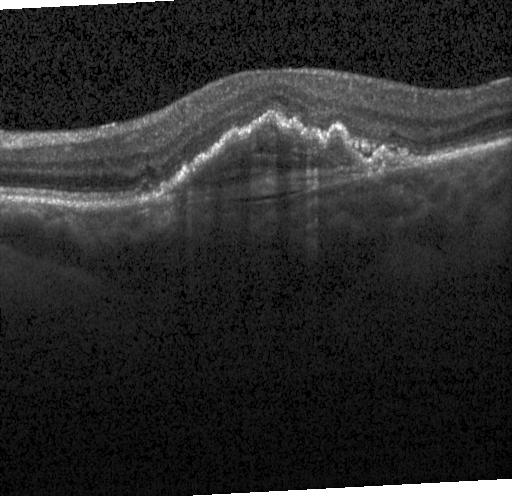

Assessment: choroidal neovascularization (CNV).